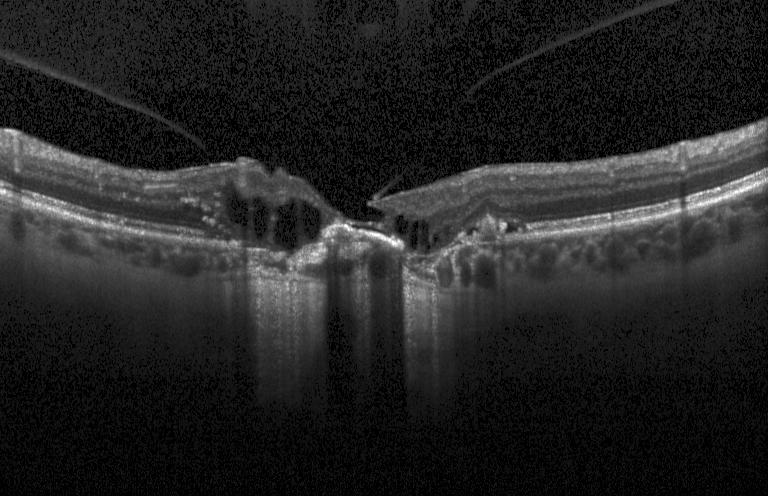
Spectral-domain OCT; fovea-centered; acquired on a Heidelberg Spectralis; retinal OCT B-scan
Diagnosis: choroidal neovascularization (CNV).